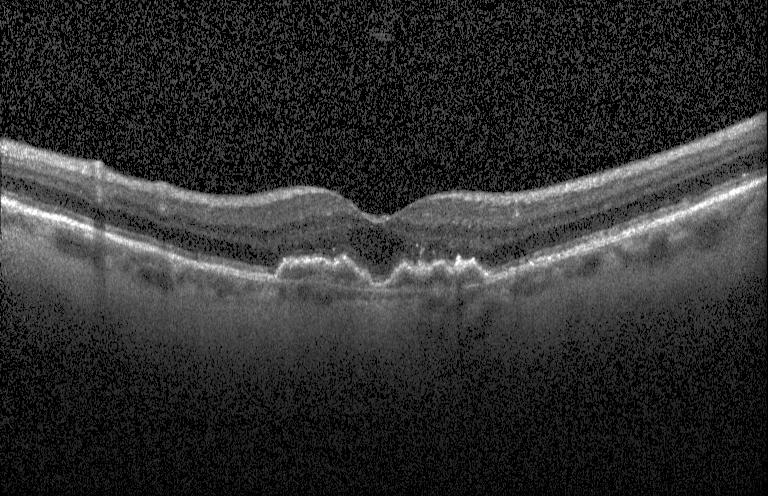 Optical coherence tomography scan. Macular scan. SD-OCT. This B-scan demonstrates choroidal neovascularization (CNV).